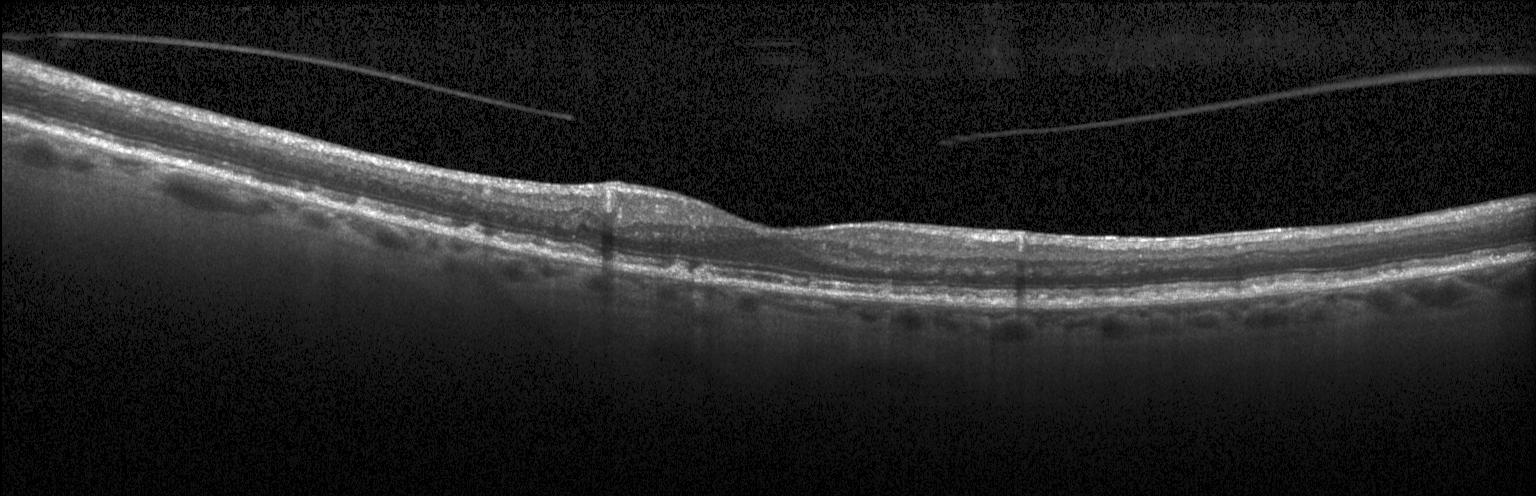

OCT B-scan · Heidelberg Spectralis · spectral-domain OCT
Diagnosis: sub-RPE drusenoid deposits.